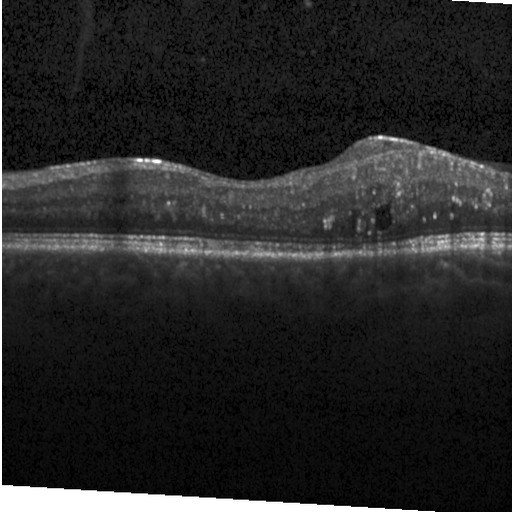
Optical coherence tomography scan — Macular OCT: DME.